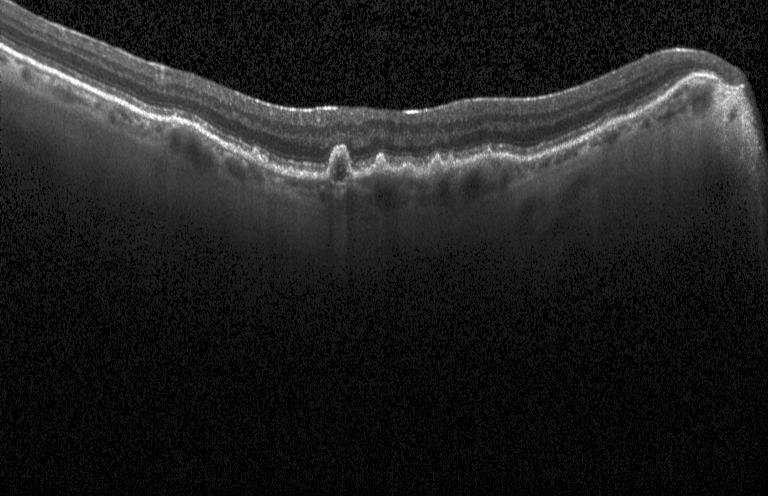 Heidelberg Spectralis. Optical coherence tomography scan.
Impression: sub-RPE drusenoid deposits.